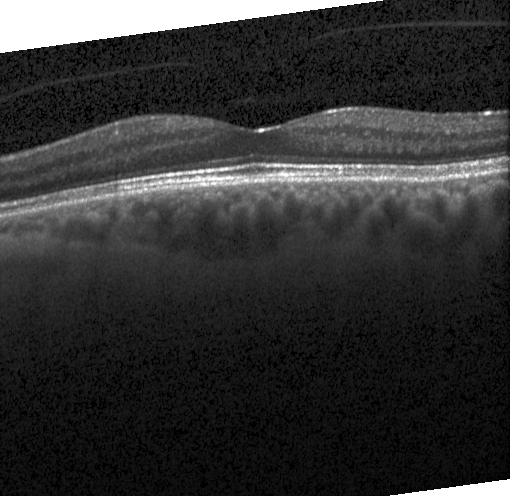
OCT line scan, instrument: Heidelberg Spectralis, spectral-domain OCT. Macular OCT: neither choroidal neovascularization, diabetic macular edema, nor drusen.